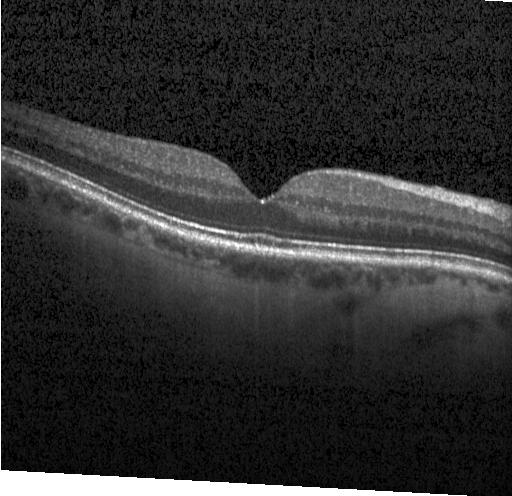

Dx: no choroidal neovascularization, no diabetic macular edema, and no drusen.